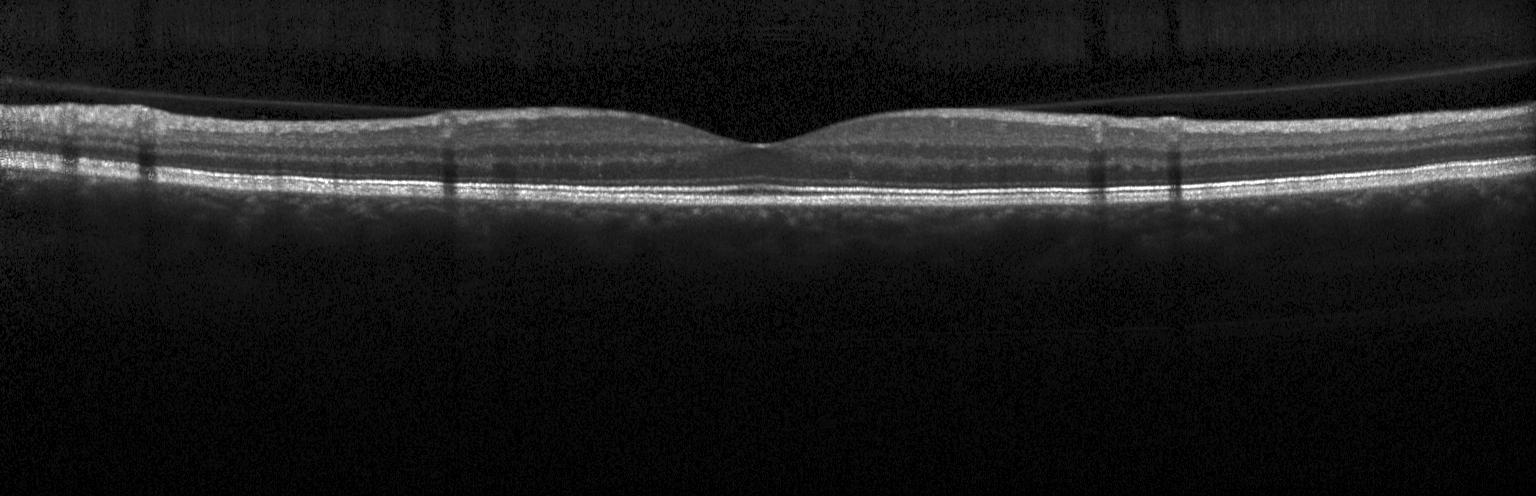 SD-OCT · OCT B-scan — Diagnosis: no evidence of CNV, DME, or drusen.